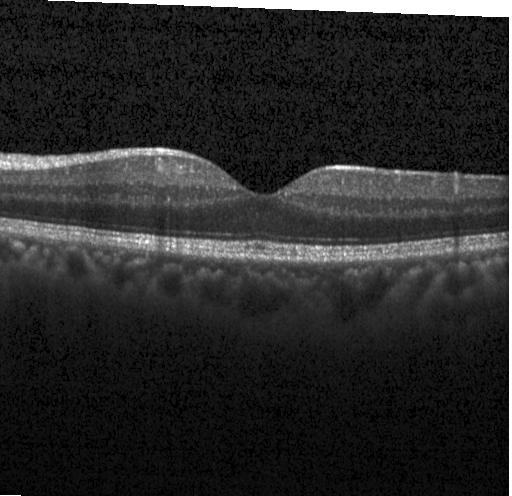
SD-OCT. Heidelberg Spectralis. Through the macula. Optical coherence tomography B-scan. Neither choroidal neovascularization, diabetic macular edema, nor drusen.